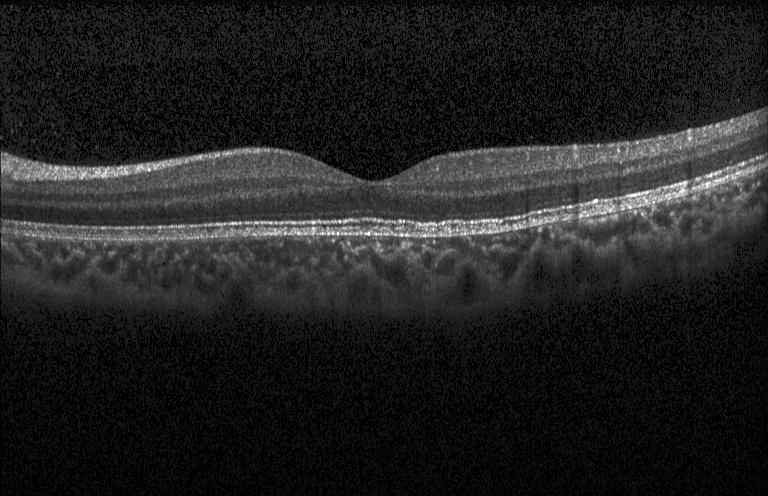

Acquired on a Heidelberg Spectralis · spectral-domain OCT · centered on the fovea · optical coherence tomography scan — Macular OCT: neither choroidal neovascularization, diabetic macular edema, nor drusen.